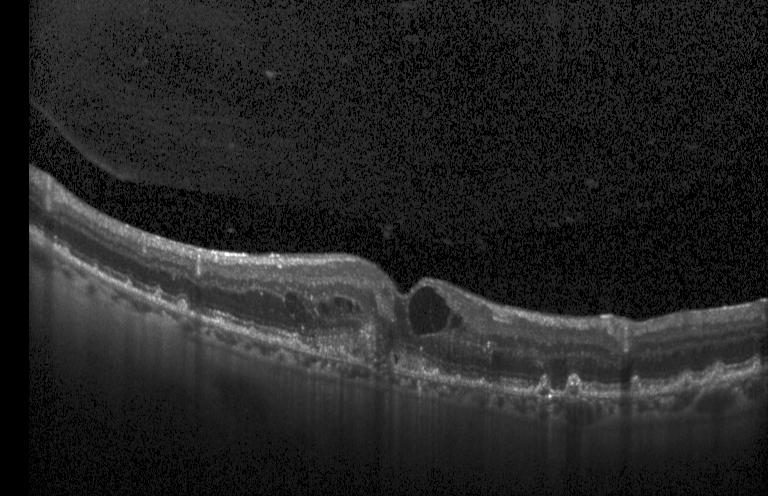 Through the macula. Spectral-domain optical coherence tomography. Optical coherence tomography B-scan. Heidelberg Spectralis OCT system. A choroidal neovascular membrane.